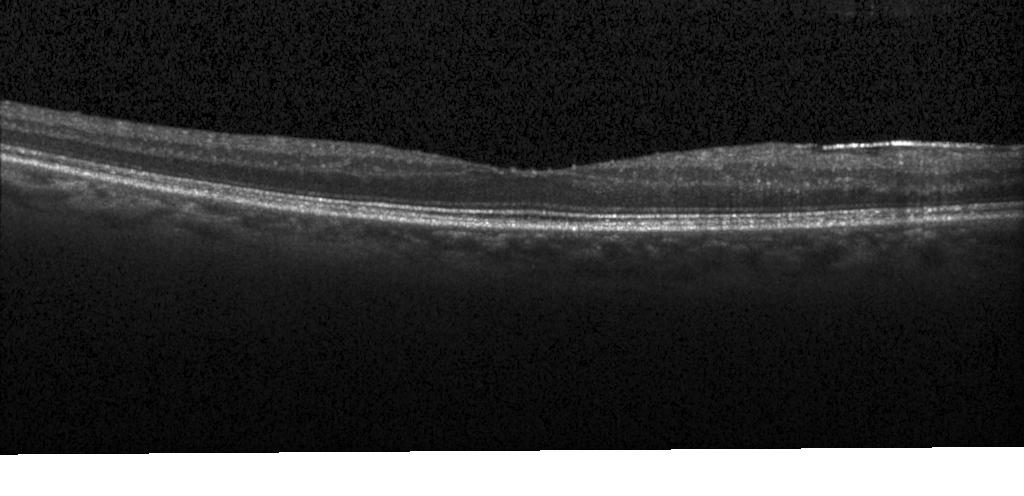 This B-scan demonstrates no evidence of choroidal neovascularization, diabetic macular edema, or drusen.